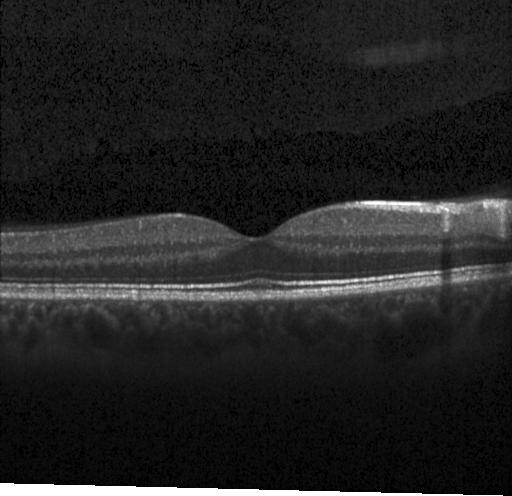 Optical coherence tomography B-scan; Heidelberg Spectralis; horizontal scan through the fovea.
Assessment: no evidence of choroidal neovascularization, diabetic macular edema, or drusen.